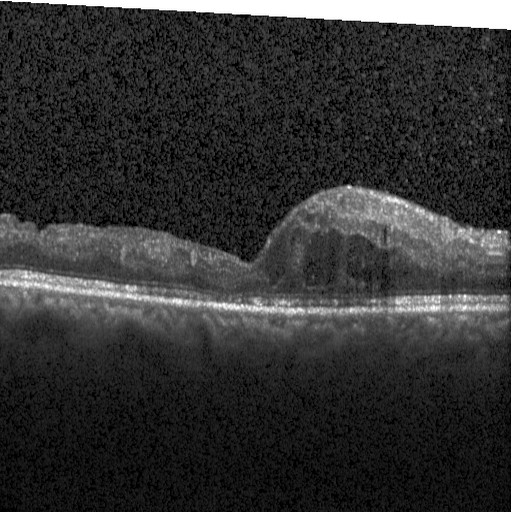
Diagnosis: DME.